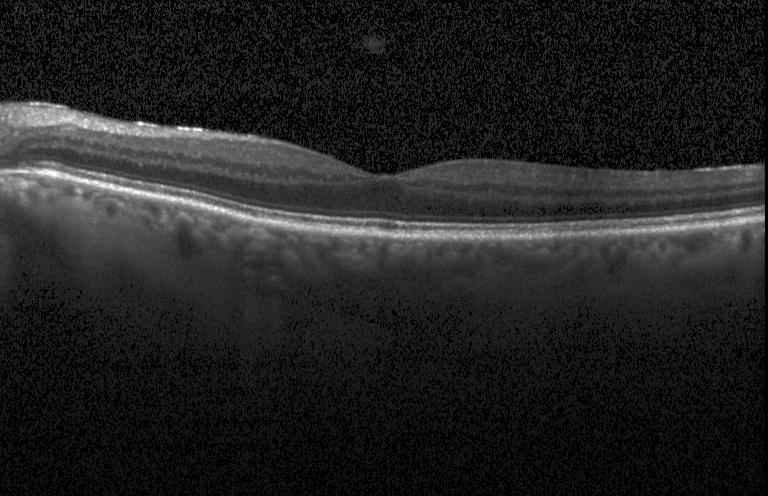
Optical coherence tomography B-scan. No CNV, no DME, and no drusen.